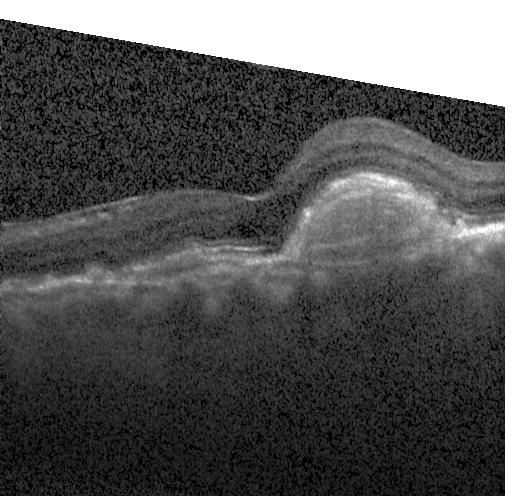 Macular OCT demonstrating a choroidal neovascular membrane.